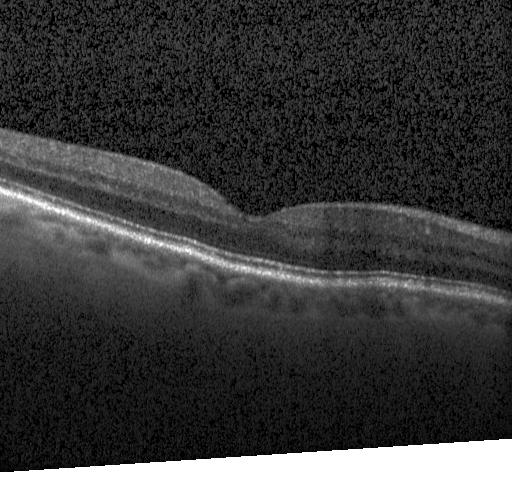 Spectral-domain optical coherence tomography, optical coherence tomography scan, fovea-centered.
Diagnosis: no choroidal neovascularization, no diabetic macular edema, and no drusen.